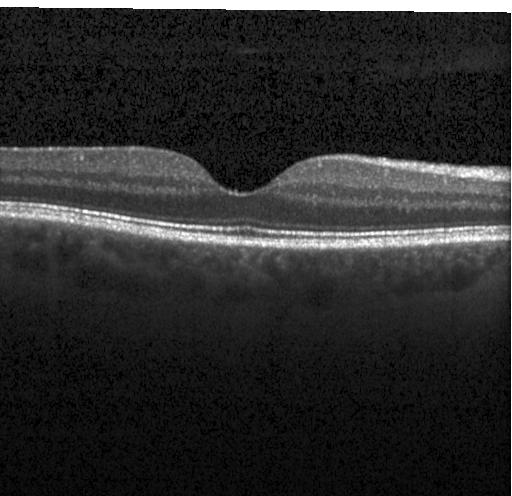

Fovea-centered, optical coherence tomography B-scan
Impression: neither choroidal neovascularization, diabetic macular edema, nor drusen.